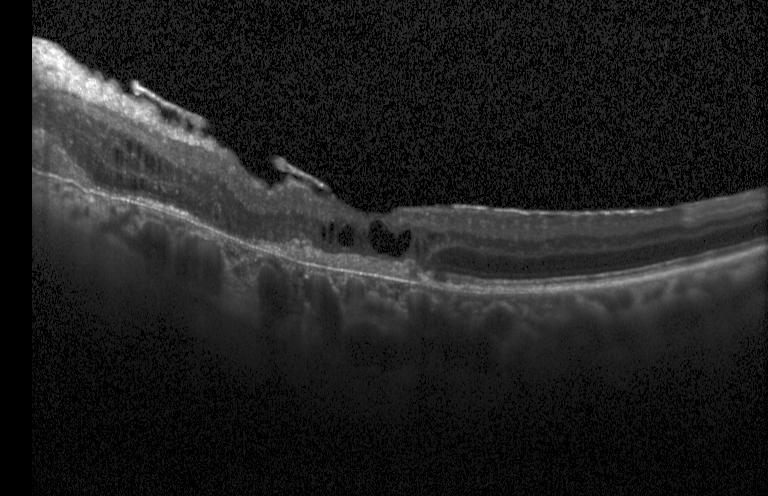
OCT B-scan. Spectral-domain OCT.
Finding: a choroidal neovascular membrane.